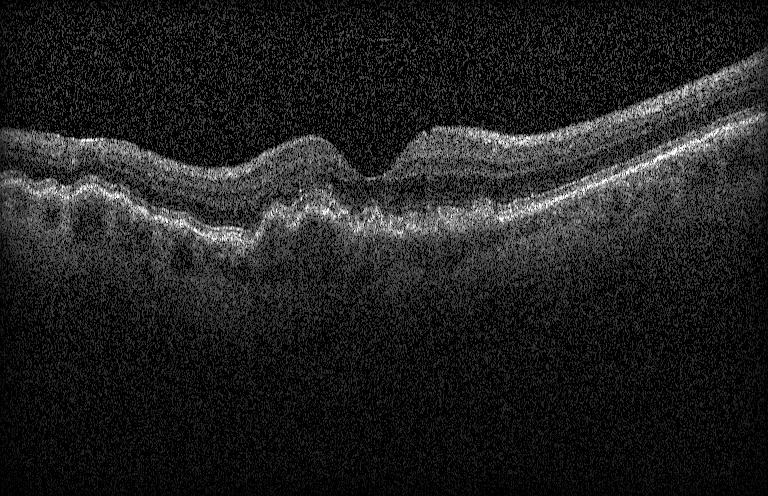

OCT B-scan showing a choroidal neovascular membrane.